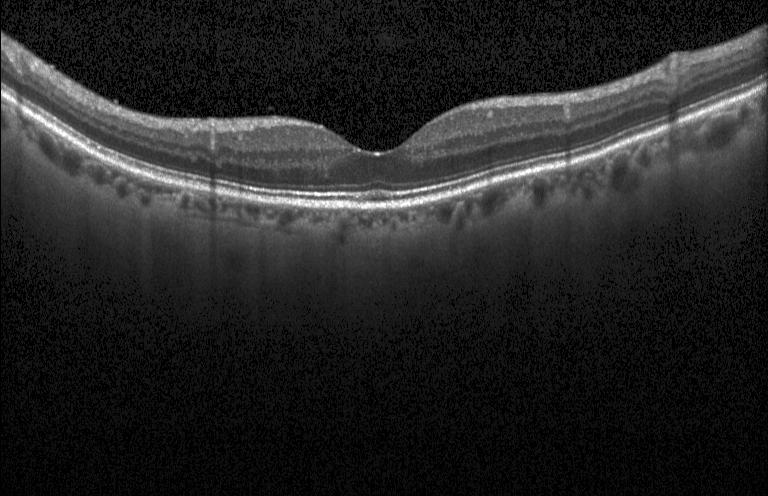 OCT B-scan. Spectral-domain optical coherence tomography. Instrument: Heidelberg Spectralis. Diagnosis: neither choroidal neovascularization, diabetic macular edema, nor drusen.